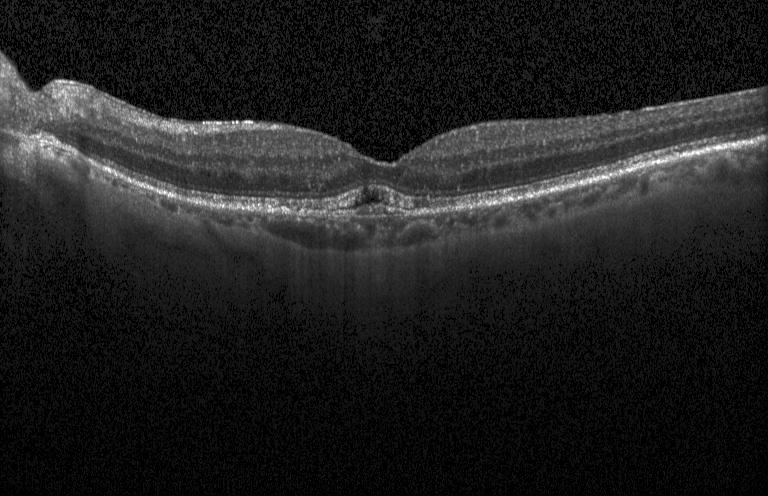

OCT line scan — Diagnosis: CNV.